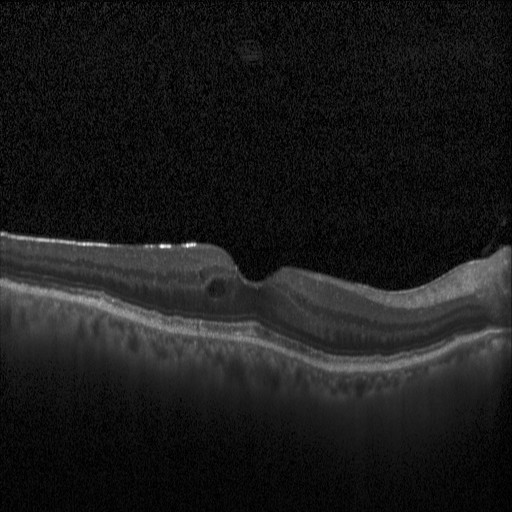 Through the macula; OCT B-scan; spectral-domain optical coherence tomography.
Dx: diabetic macular edema.